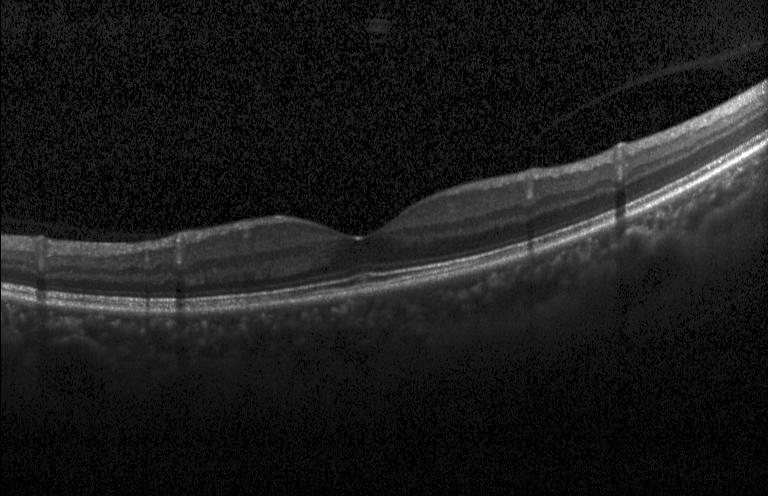

Horizontal scan through the fovea; optical coherence tomography scan; Heidelberg Spectralis.
The scan shows no choroidal neovascularization, diabetic macular edema, or drusen.